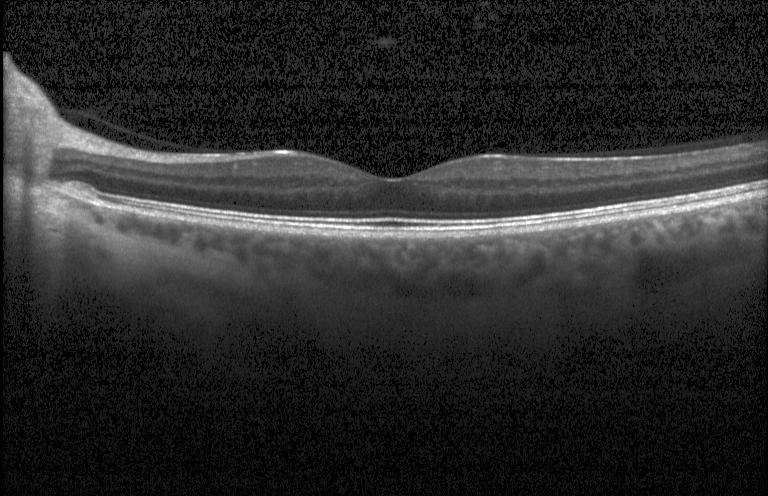 Macular OCT: no evidence of choroidal neovascularization, diabetic macular edema, or drusen.